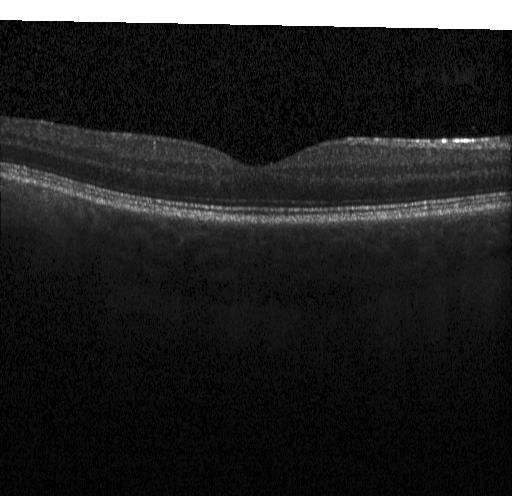

OCT B-scan
Macular OCT: no choroidal neovascularization, diabetic macular edema, or drusen.